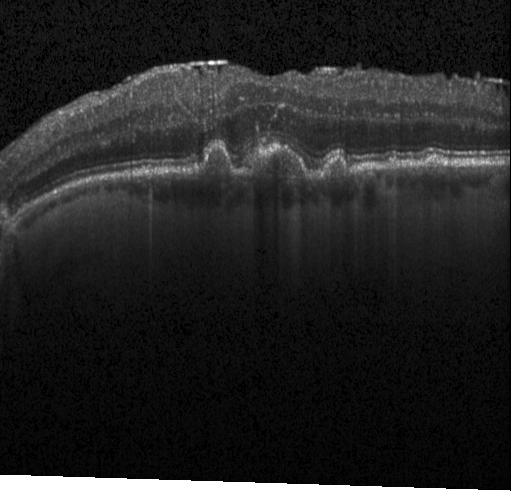 OCT line scan — Diagnosis: drusen.